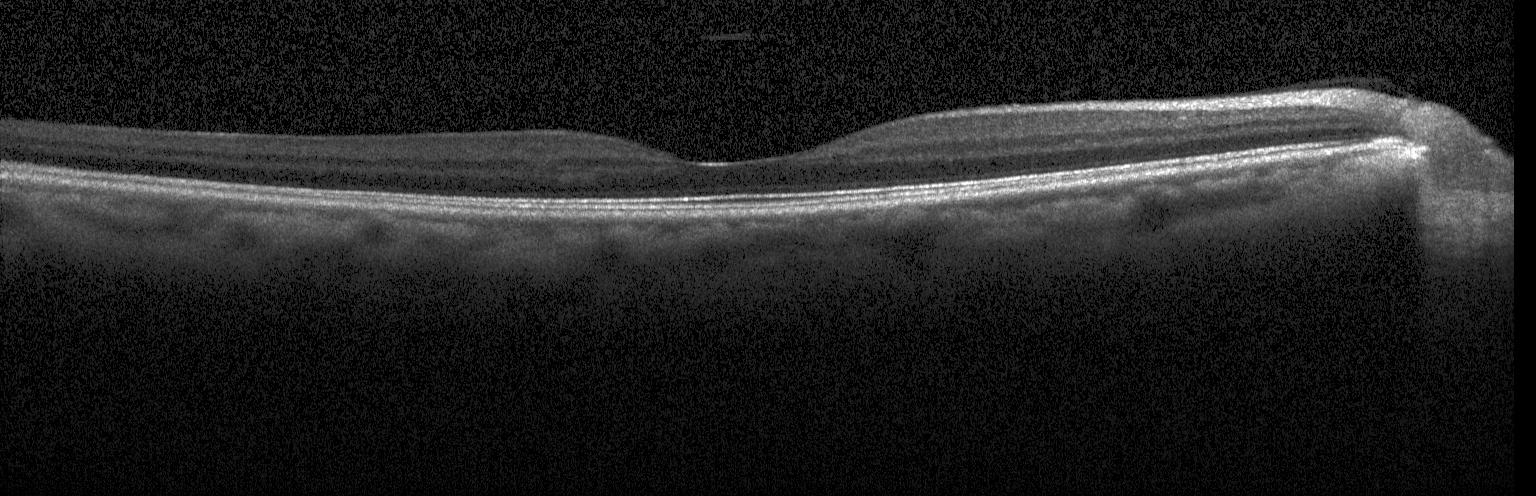 OCT line scan. Heidelberg Spectralis OCT system. Spectral-domain OCT
Impression: no choroidal neovascularization, no diabetic macular edema, and no drusen.